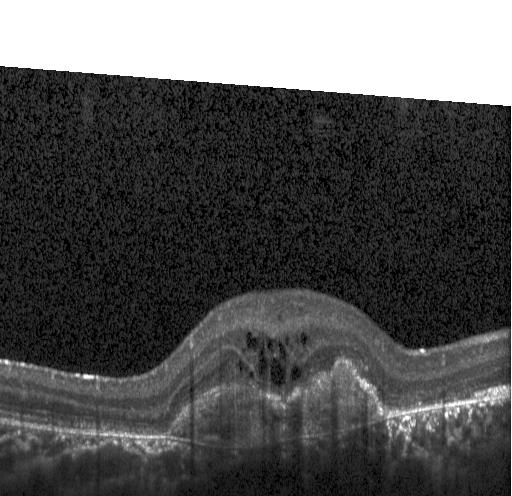

Optical coherence tomography scan; spectral-domain optical coherence tomography; acquired on a Heidelberg Spectralis
The scan shows a choroidal neovascular membrane.